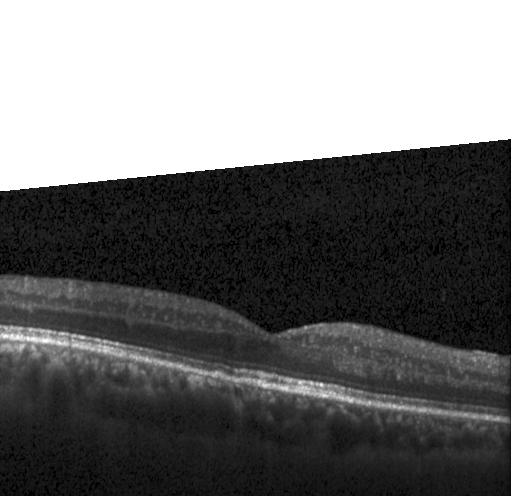
Retinal OCT cross-section showing neither choroidal neovascularization, diabetic macular edema, nor drusen.